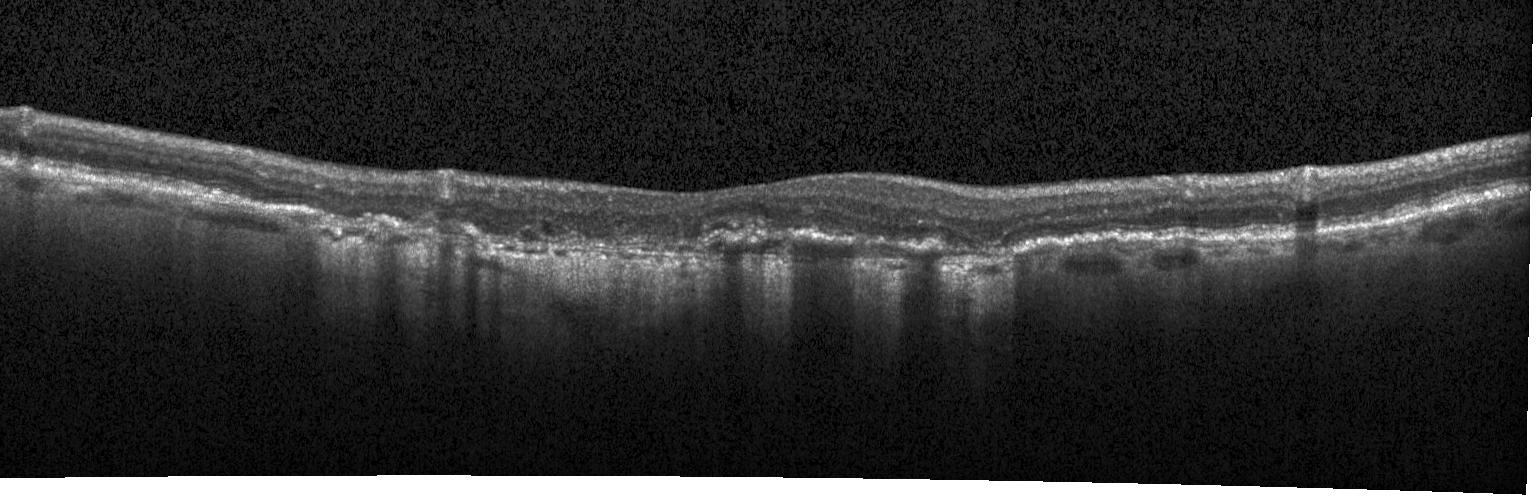

Optical coherence tomography scan; Heidelberg Spectralis OCT system — This B-scan demonstrates a choroidal neovascular membrane.